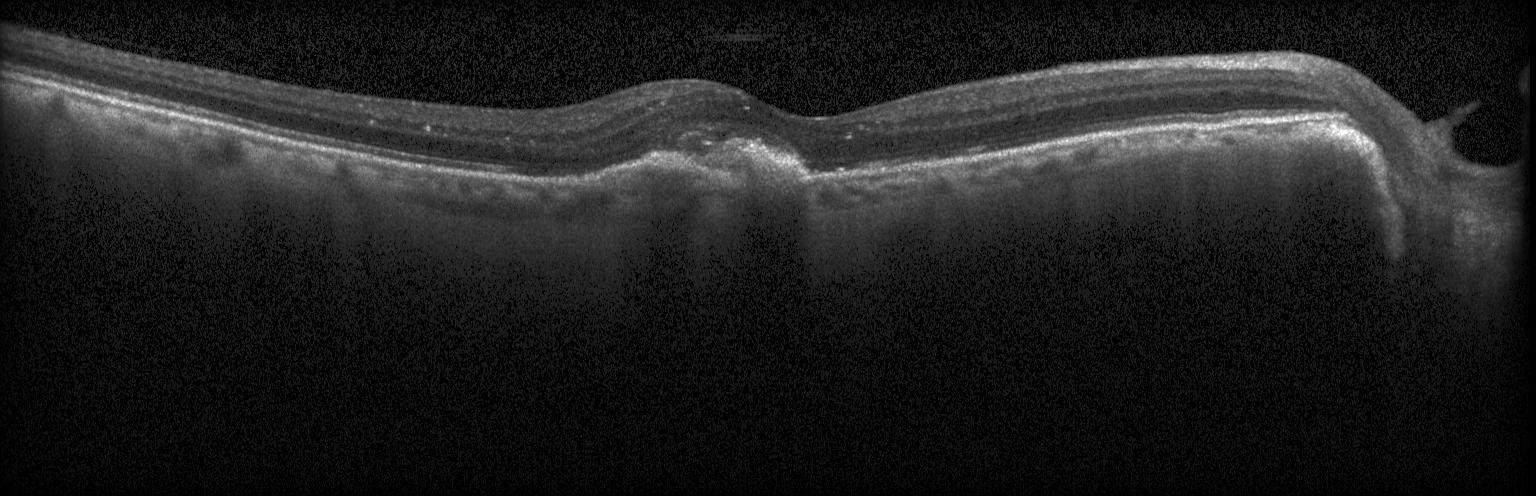
Impression: choroidal neovascularization.